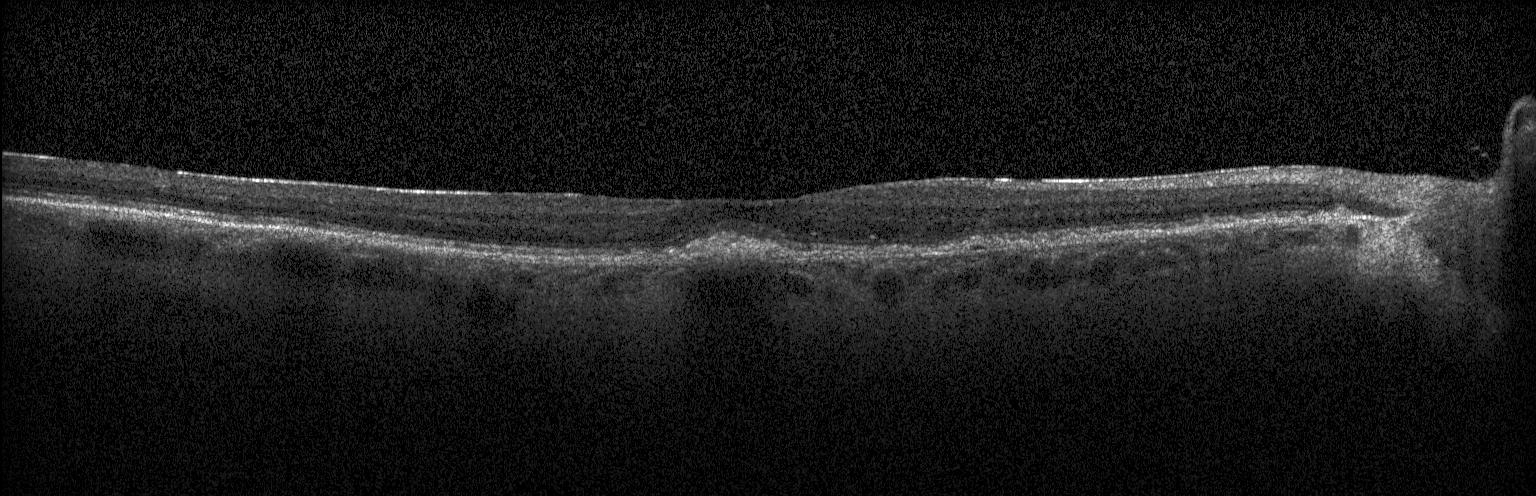

Centered on the fovea; spectral-domain optical coherence tomography; retinal OCT B-scan; Heidelberg Spectralis — Macular OCT: choroidal neovascularization.